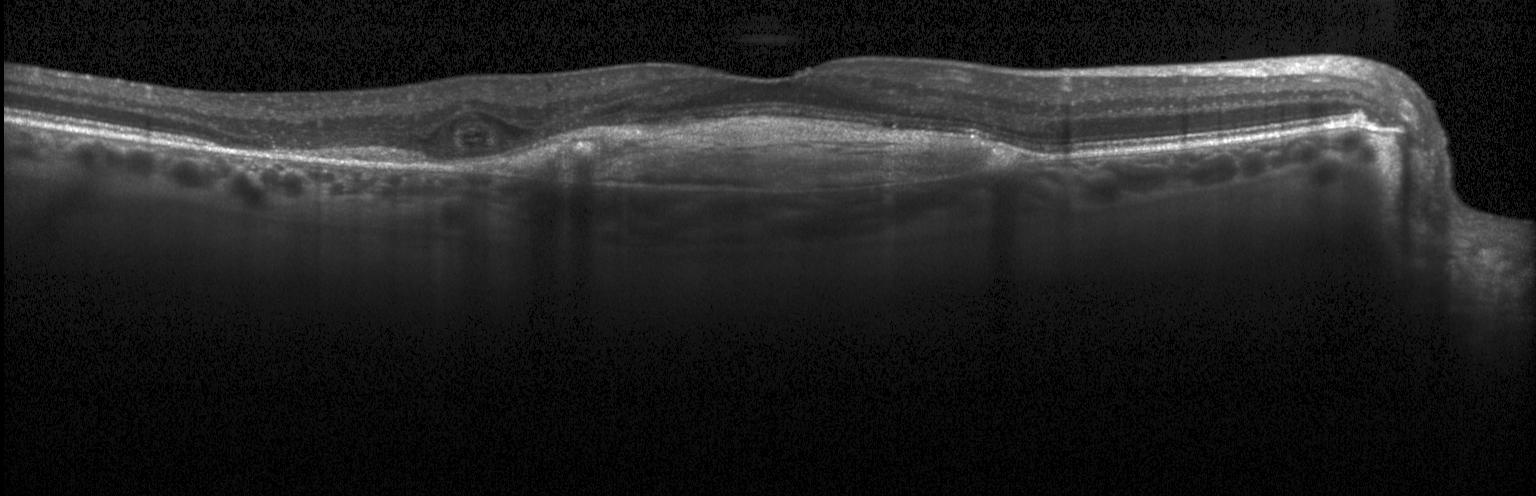
Dx: choroidal neovascularization (CNV).